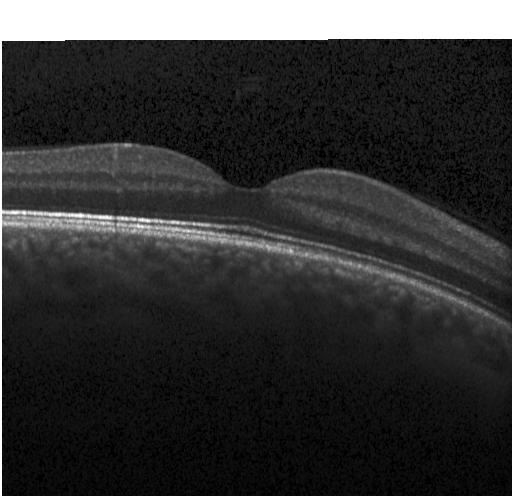

Finding: no choroidal neovascularization, no diabetic macular edema, and no drusen.